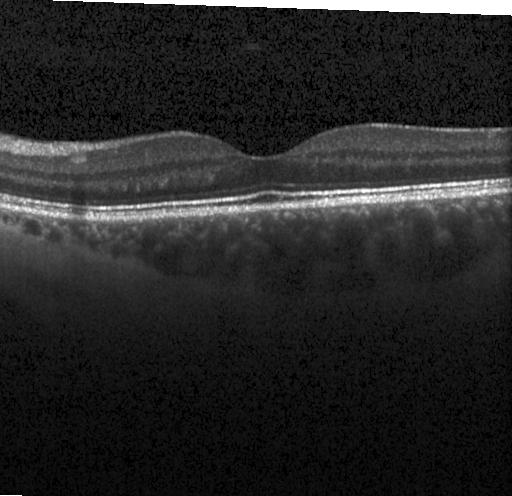
OCT scan showing no choroidal neovascularization, no diabetic macular edema, and no drusen.